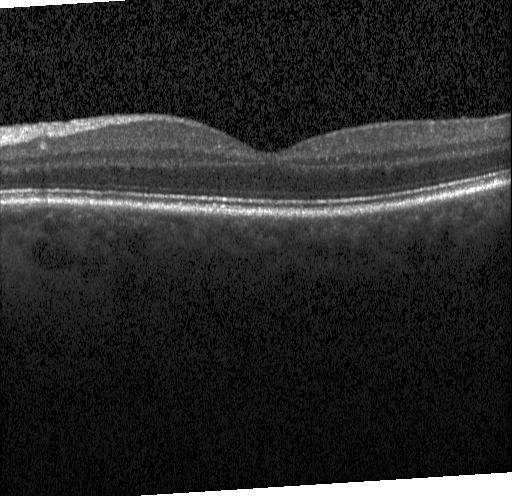

This B-scan demonstrates no choroidal neovascularization, no diabetic macular edema, and no drusen.